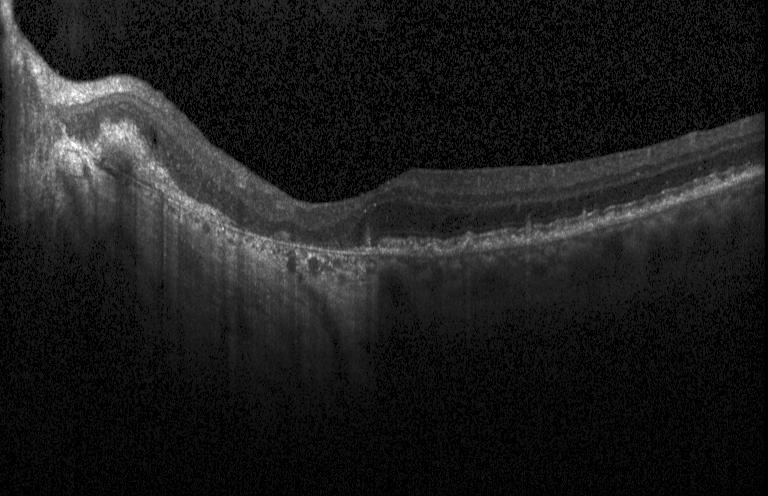
Heidelberg Spectralis OCT system; centered on the fovea; optical coherence tomography B-scan. Diagnosis: CNV.